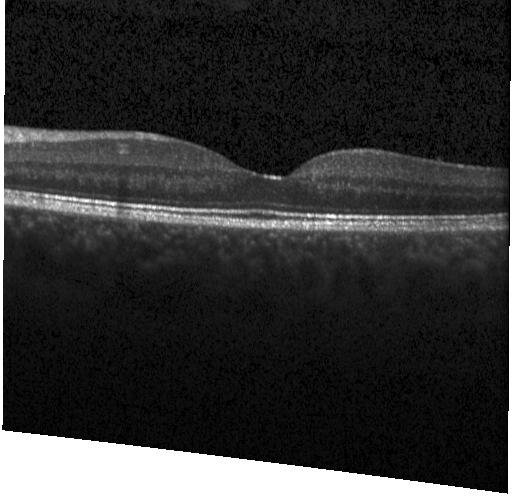 Acquired on a Heidelberg Spectralis · OCT line scan — Impression: no choroidal neovascularization, no diabetic macular edema, and no drusen.